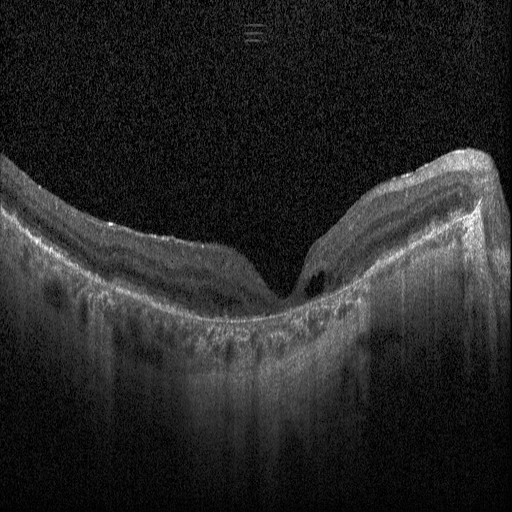
Spectral-domain OCT · OCT B-scan · Heidelberg Spectralis. OCT finding: diabetic macular edema (DME).